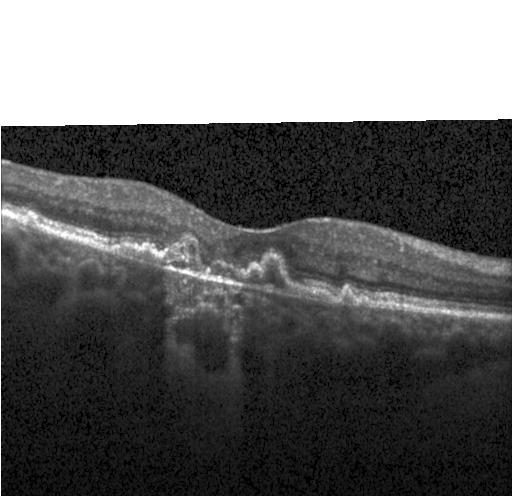
OCT B-scan, centered on the fovea, spectral-domain OCT. Impression: a choroidal neovascular membrane.